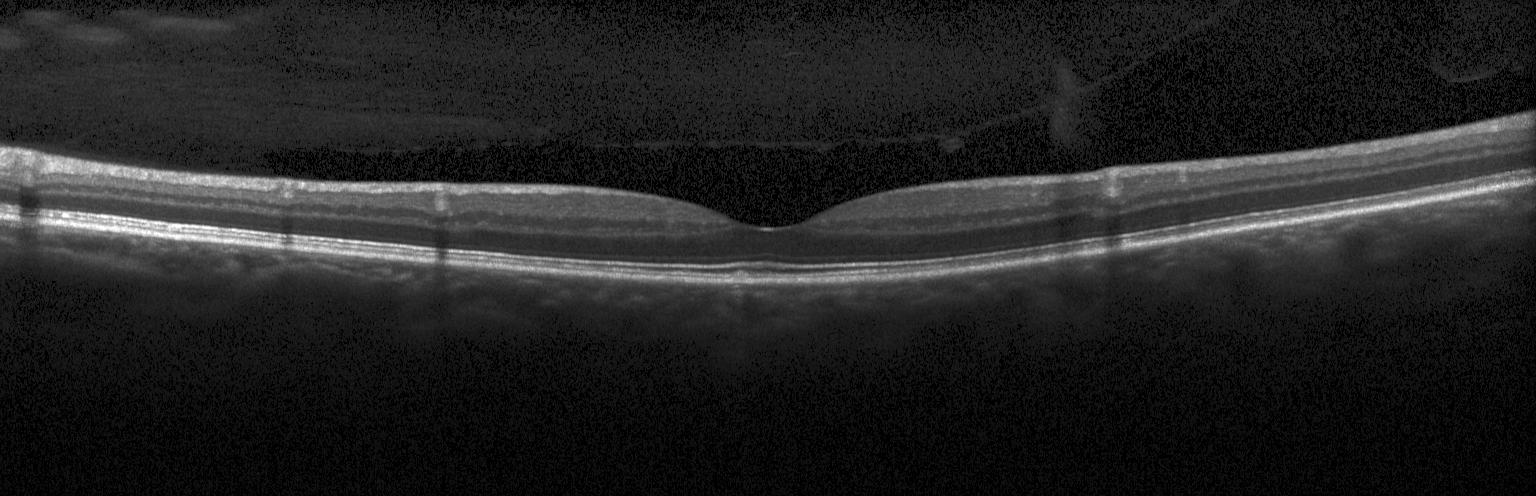

Heidelberg Spectralis OCT system; optical coherence tomography B-scan — No choroidal neovascularization, no diabetic macular edema, and no drusen.